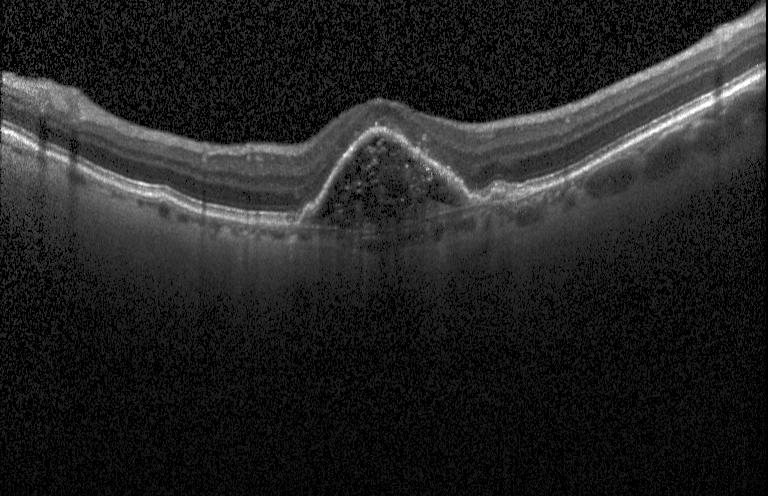

Heidelberg Spectralis; optical coherence tomography B-scan; centered on the fovea — This B-scan demonstrates a choroidal neovascular membrane.